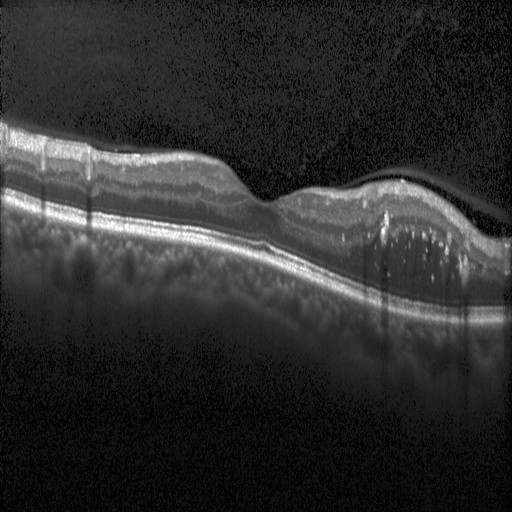
OCT finding: diabetic macular edema.